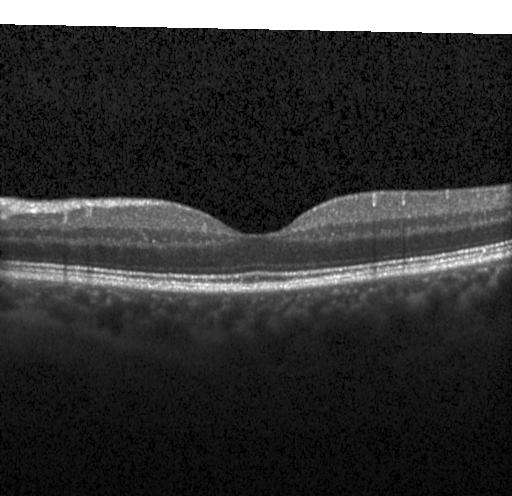 No choroidal neovascularization, diabetic macular edema, or drusen.